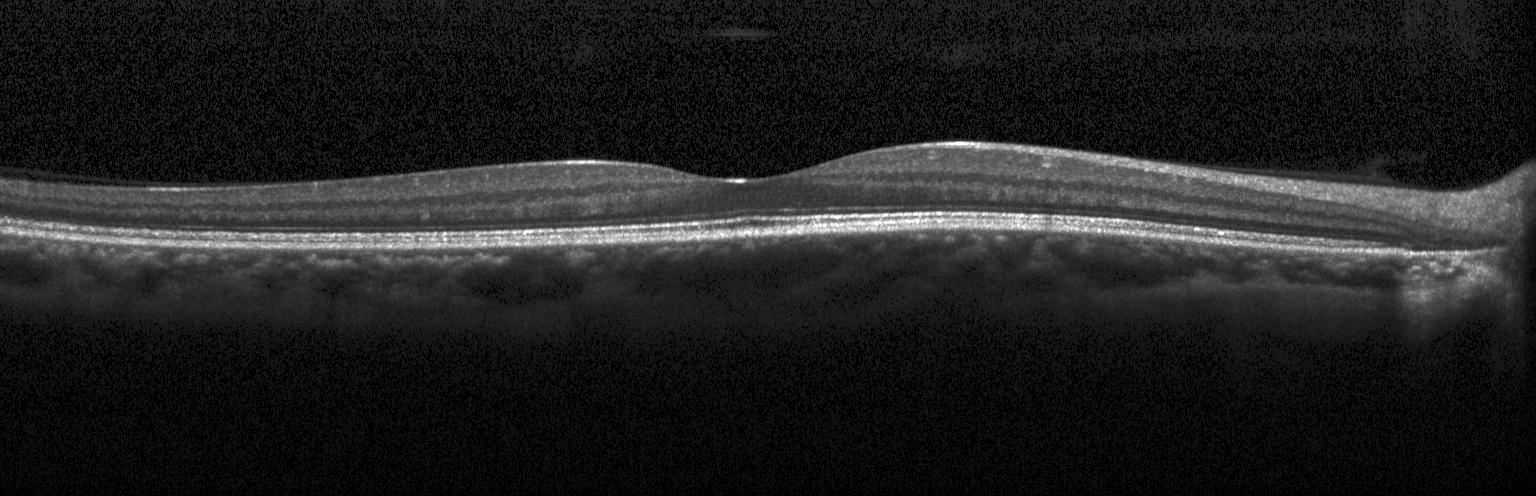

Finding: no CNV, no DME, and no drusen.